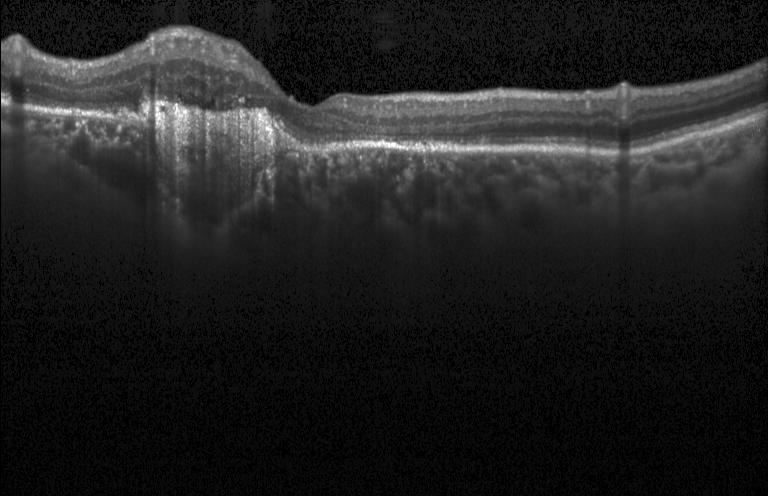 Retinal OCT B-scan
Impression: a choroidal neovascular membrane.